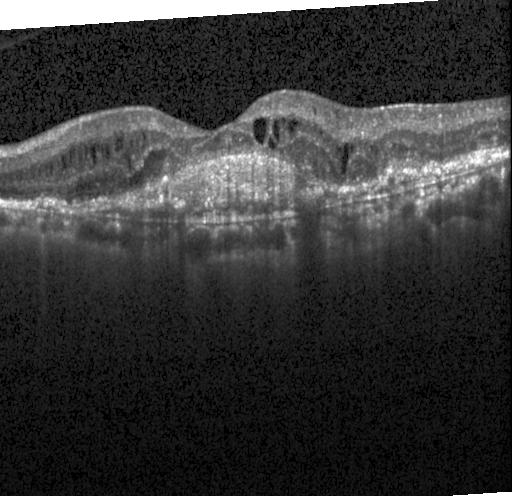
Spectral-domain OCT B-scan: choroidal neovascularization.